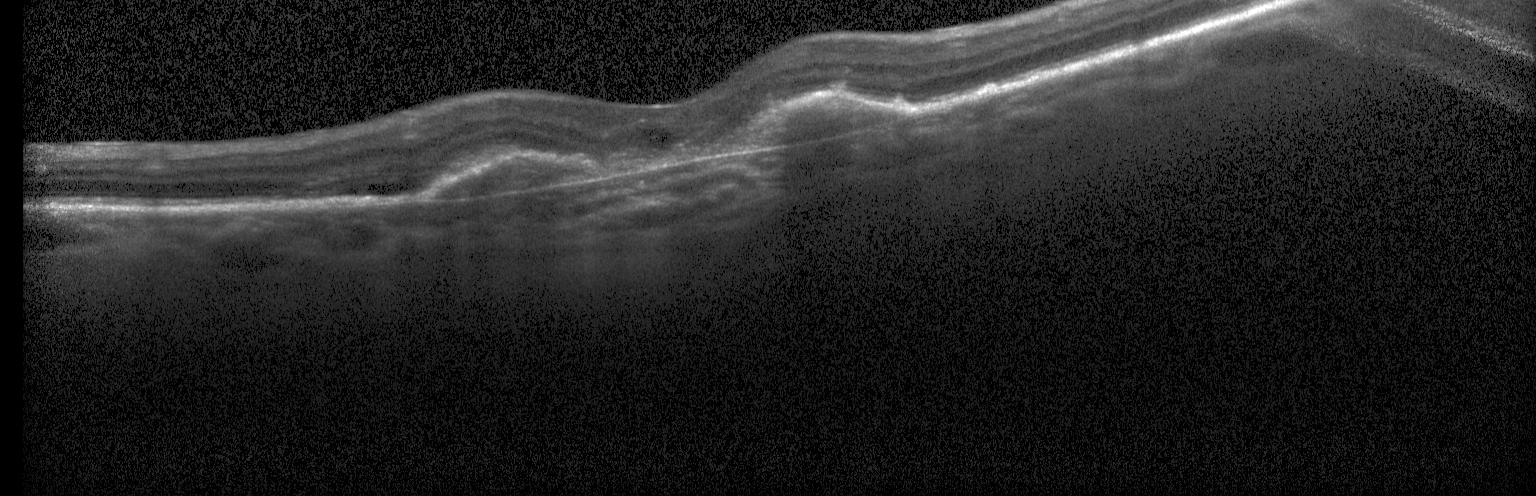
OCT finding: a choroidal neovascular membrane.